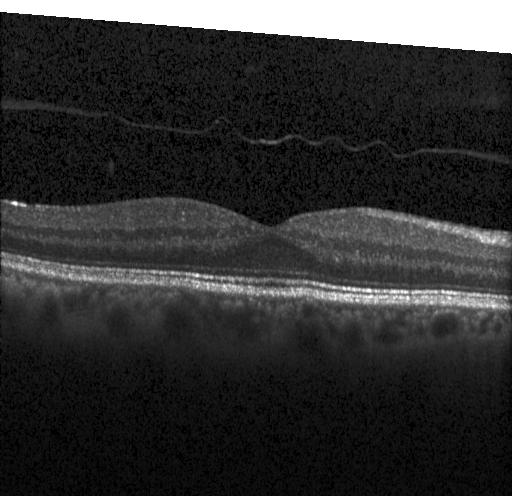
OCT finding: no choroidal neovascularization, no diabetic macular edema, and no drusen.